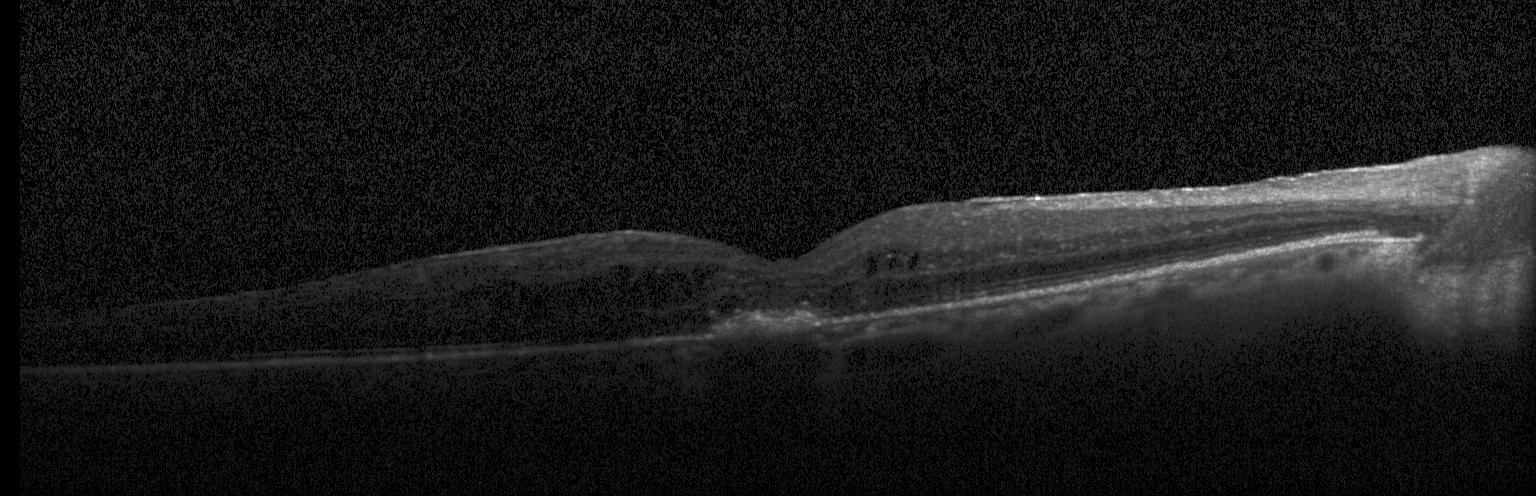
Acquired on a Heidelberg Spectralis. Through the macula. OCT B-scan. Spectral-domain optical coherence tomography.
Diagnosis: DME.